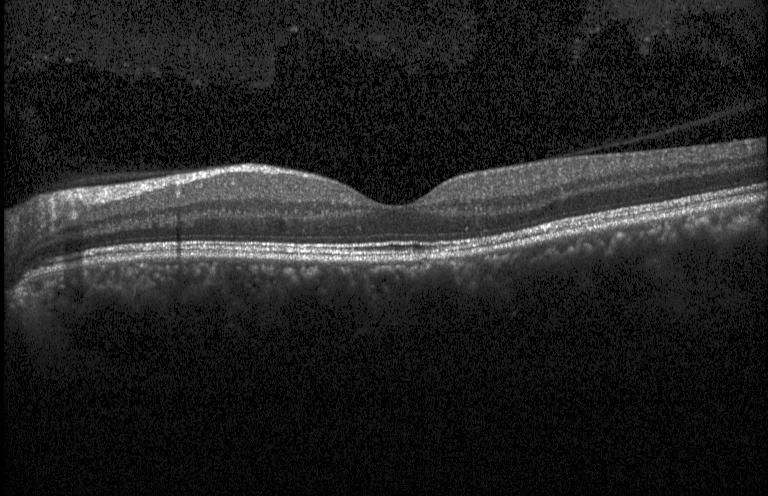 Assessment: neither choroidal neovascularization, diabetic macular edema, nor drusen.